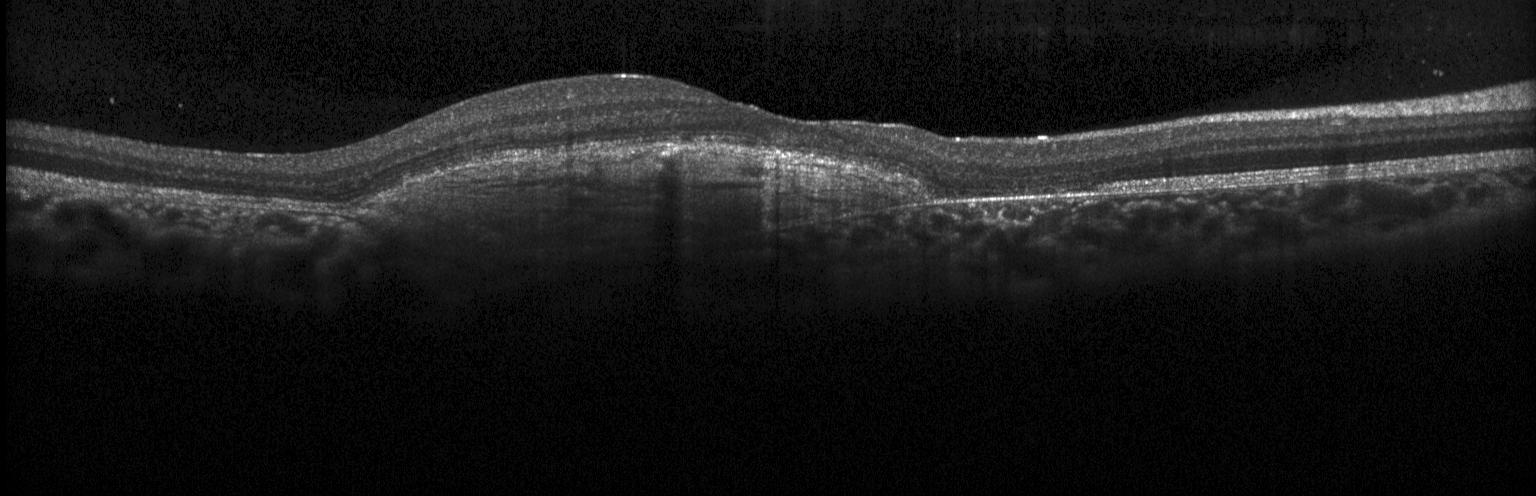 OCT line scan; fovea-centered; instrument: Heidelberg Spectralis — Impression: choroidal neovascularization.